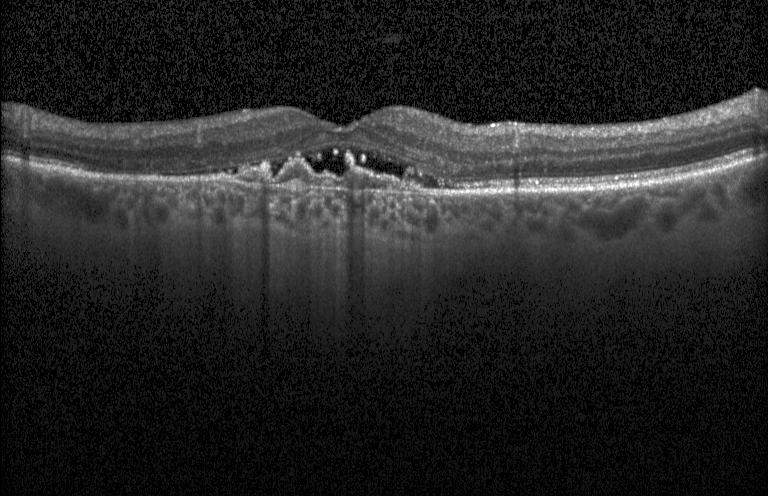

Optical coherence tomography B-scan, spectral-domain OCT, Heidelberg Spectralis, centered on the fovea. Finding: a choroidal neovascular membrane.